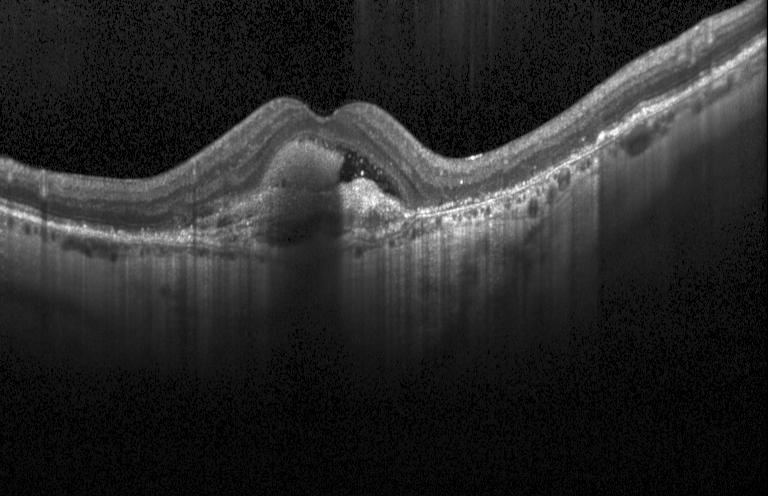
Optical coherence tomography B-scan · spectral-domain OCT · centered on the fovea — Assessment: a choroidal neovascular membrane.